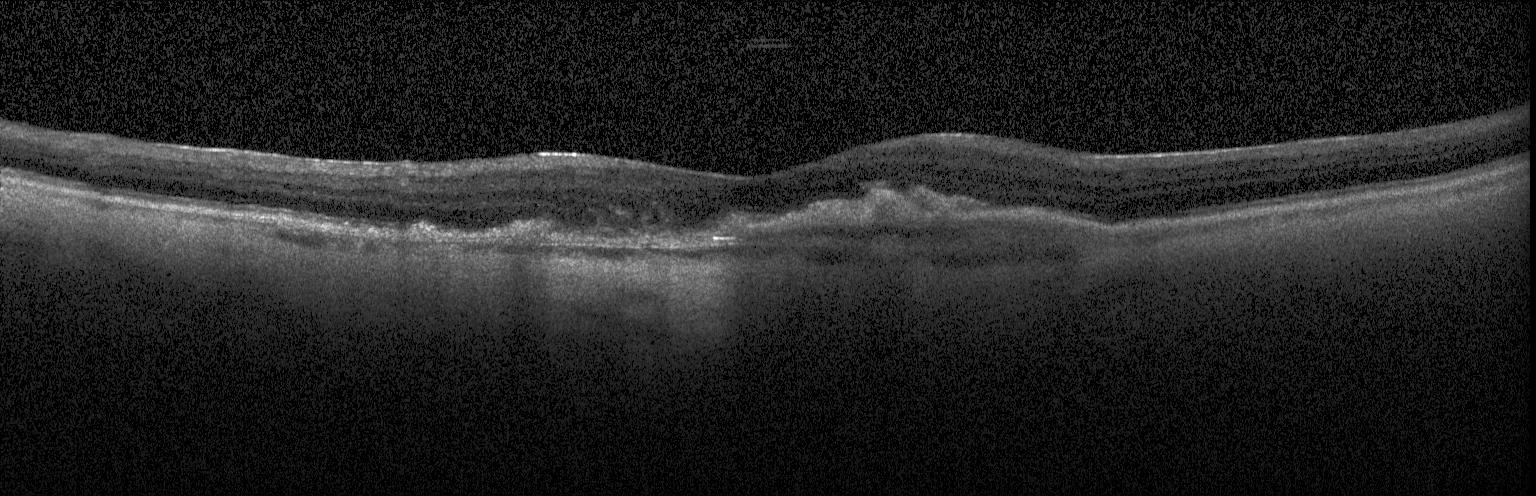
Retinal OCT cross-section showing choroidal neovascularization.